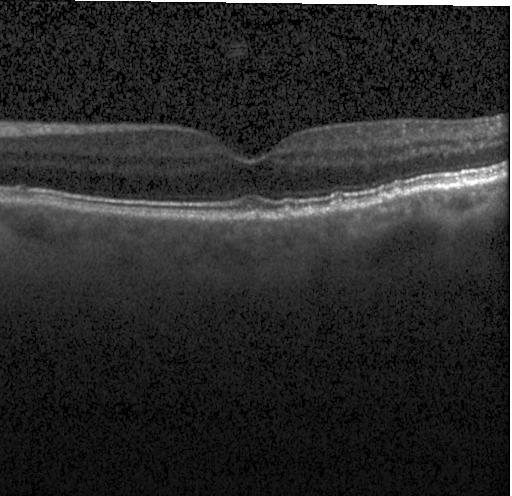 This B-scan demonstrates drusen.